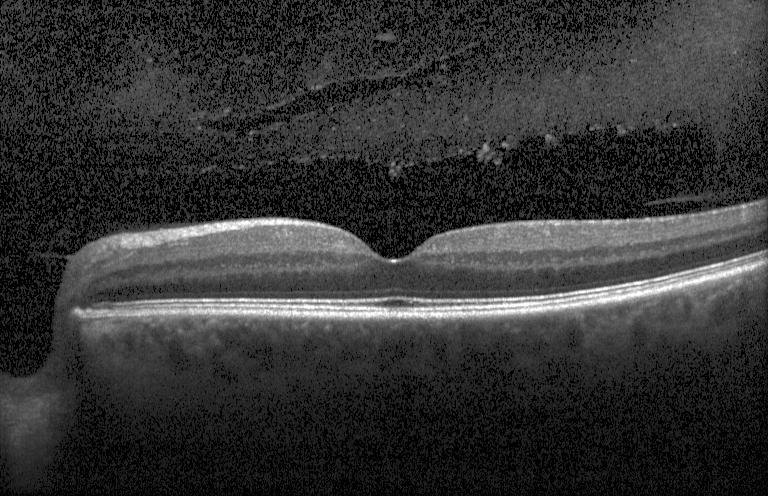

Heidelberg Spectralis · spectral-domain OCT · horizontal scan through the fovea · OCT B-scan. The scan shows neither choroidal neovascularization, diabetic macular edema, nor drusen.